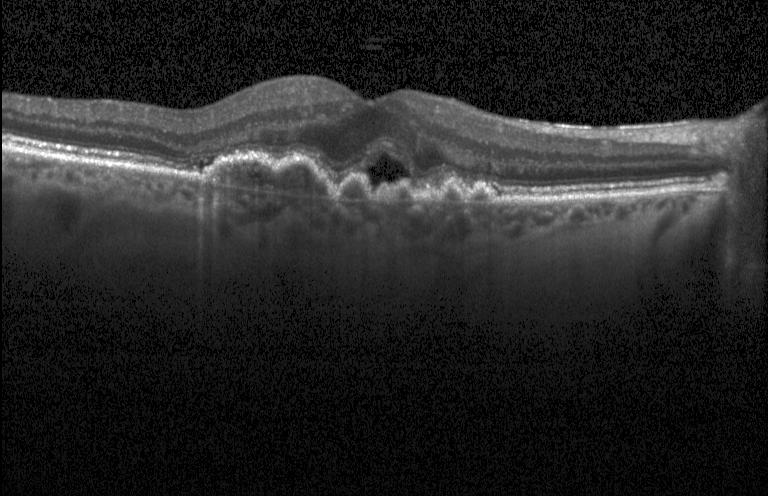
Macular scan, retinal OCT B-scan — Assessment: a choroidal neovascular membrane.